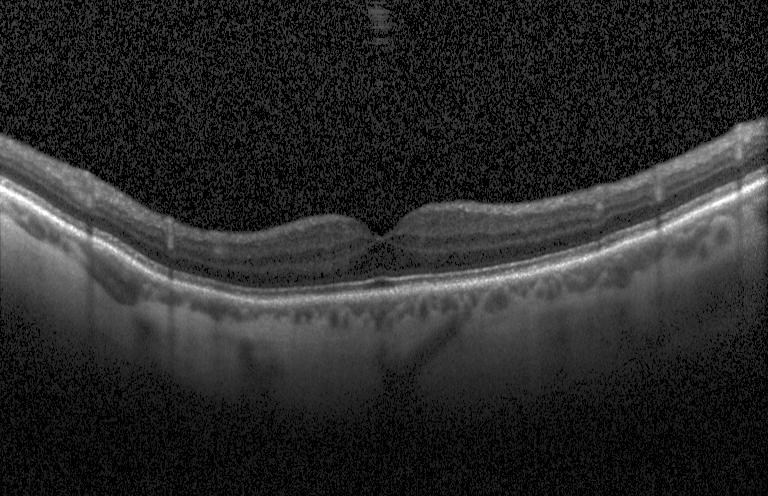 Dx: neither CNV, DME, nor drusen.